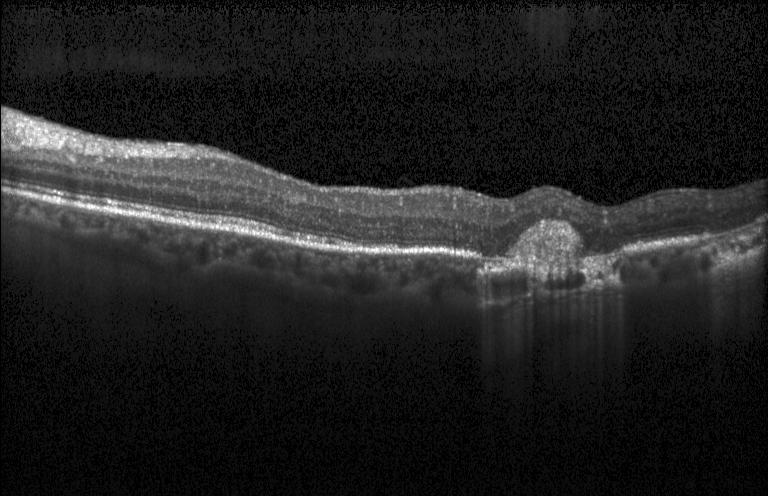 Optical coherence tomography scan. Spectral-domain optical coherence tomography. Heidelberg Spectralis. Horizontal scan through the fovea — Diagnosis: choroidal neovascularization (CNV).